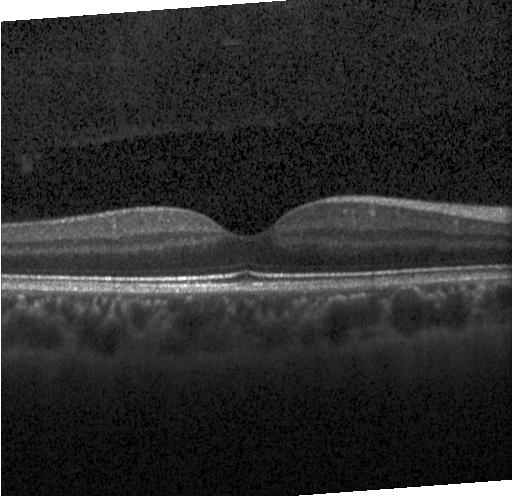

Fovea-centered. Optical coherence tomography B-scan — OCT finding: no evidence of CNV, DME, or drusen.